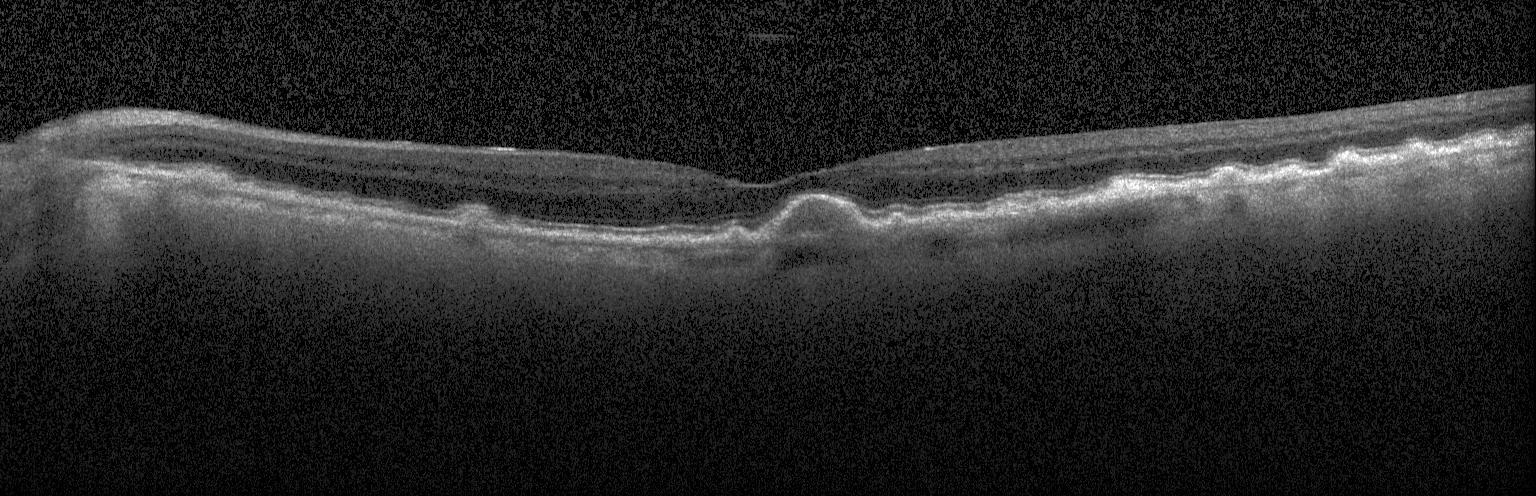 OCT B-scan
The scan shows sub-RPE drusenoid deposits.